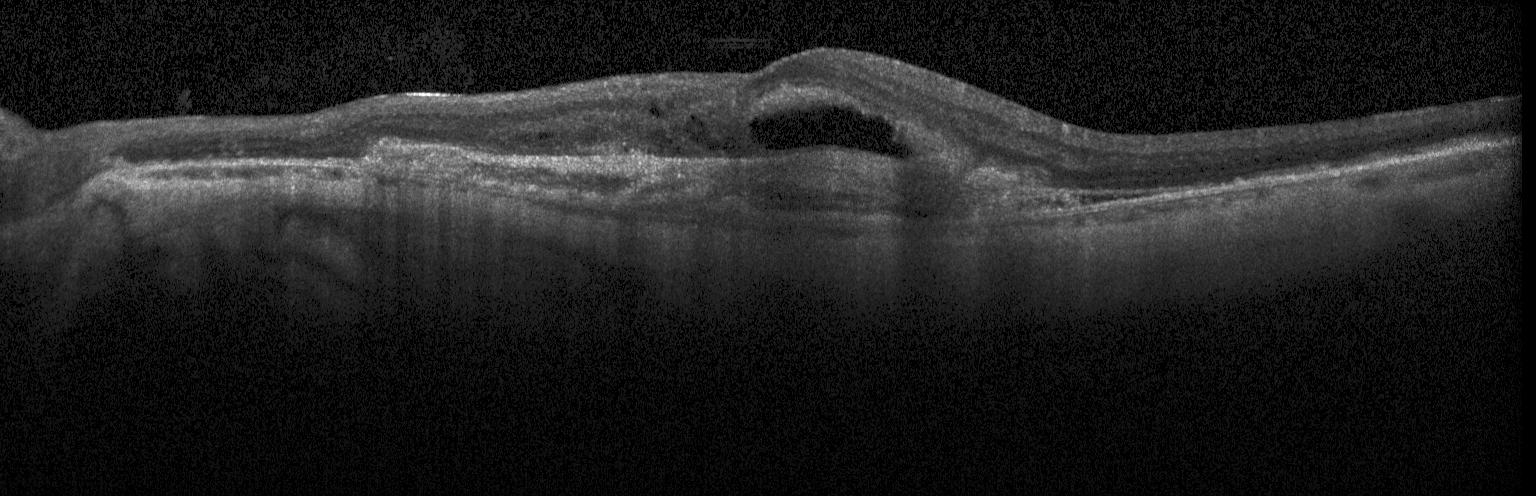
SD-OCT, OCT line scan, macular scan — Finding: choroidal neovascularization (CNV).